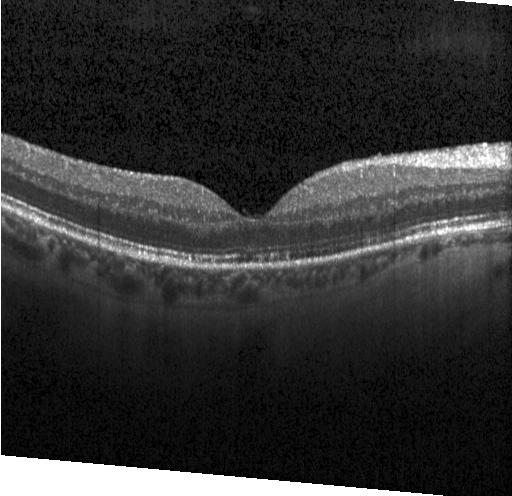

Heidelberg Spectralis OCT system. OCT B-scan. Macular scan.
Finding: no evidence of choroidal neovascularization, diabetic macular edema, or drusen.